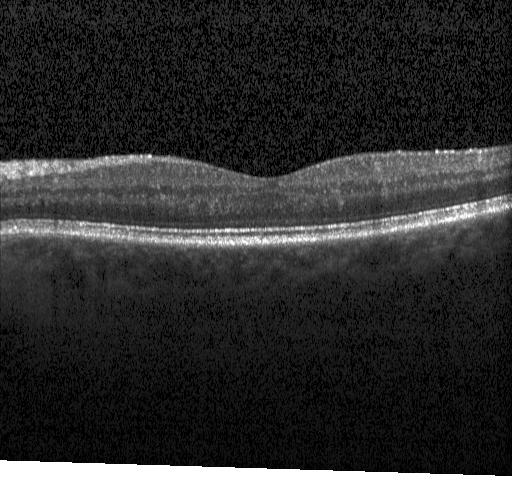
OCT line scan.
Macular OCT: no choroidal neovascularization, diabetic macular edema, or drusen.